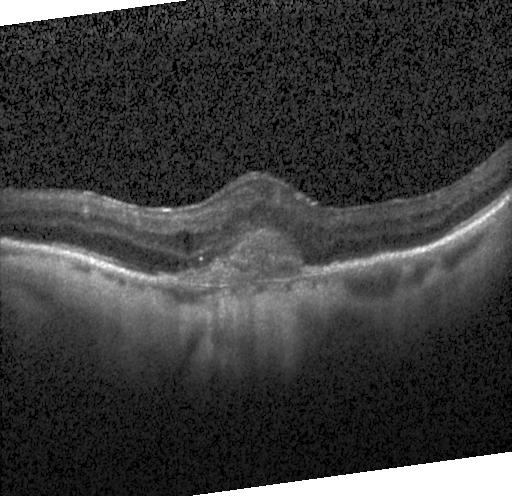

Retinal OCT cross-section showing a choroidal neovascular membrane.